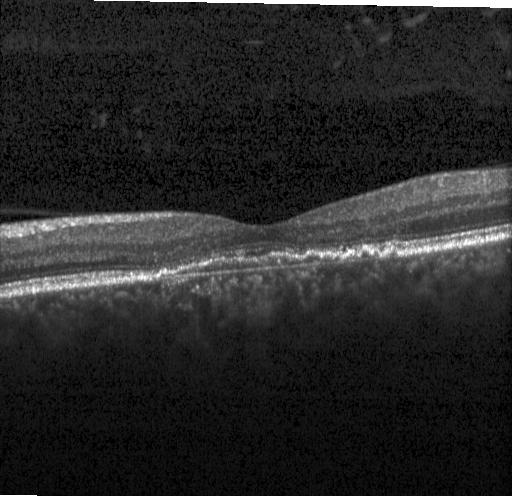 Acquired on a Heidelberg Spectralis, optical coherence tomography scan — Finding: a choroidal neovascular membrane.